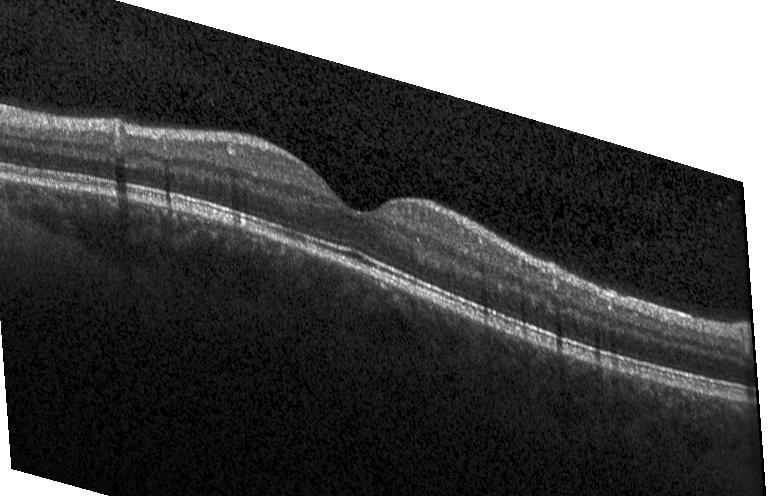

Impression: no choroidal neovascularization, no diabetic macular edema, and no drusen.